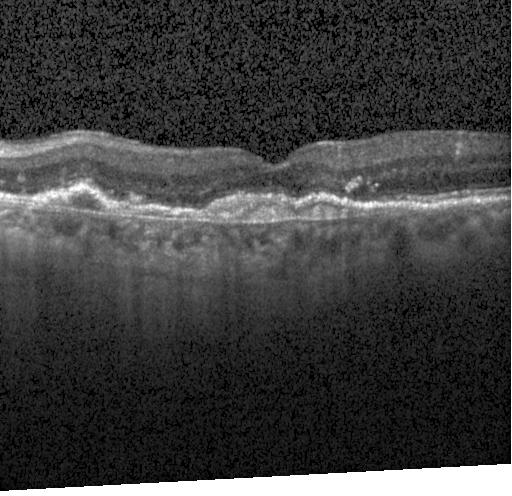

Dx: choroidal neovascularization.